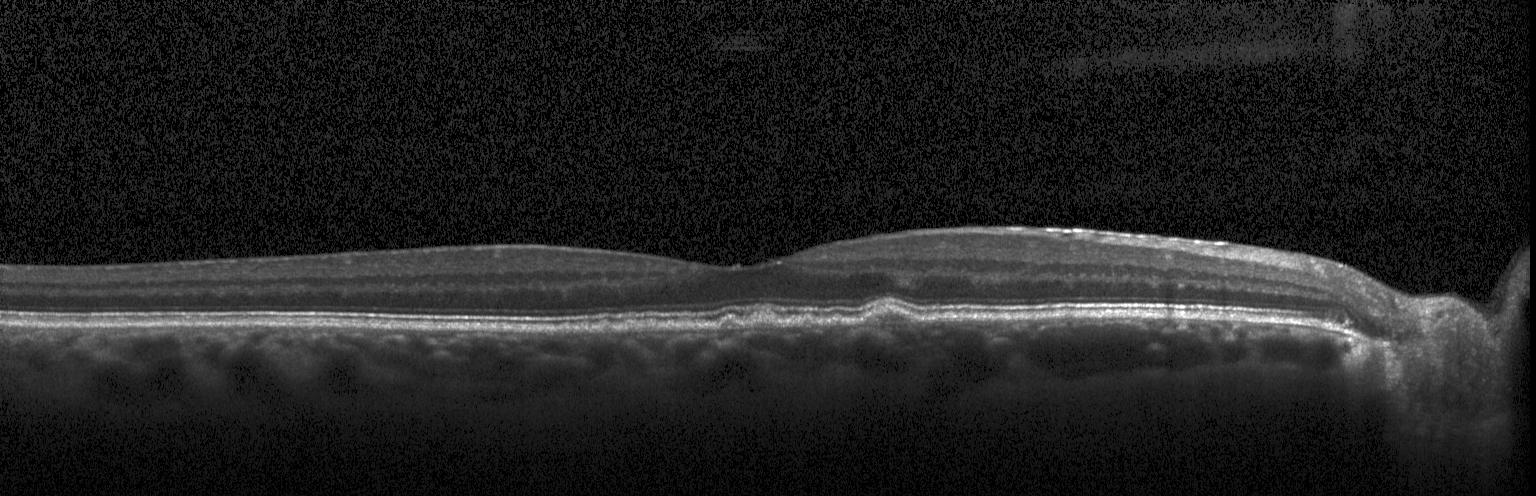 Retinal OCT cross-section showing drusen.